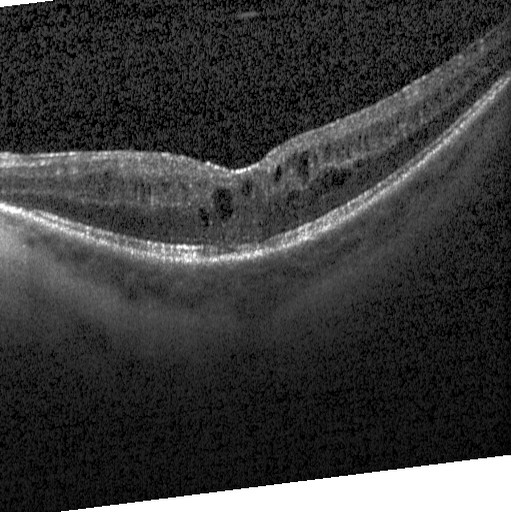

OCT line scan
Finding: diabetic macular edema (DME).